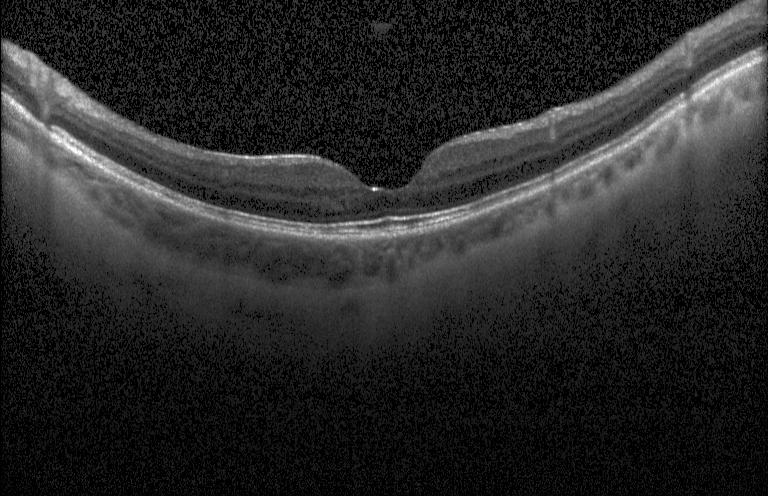 Finding: no CNV, DME, or drusen.